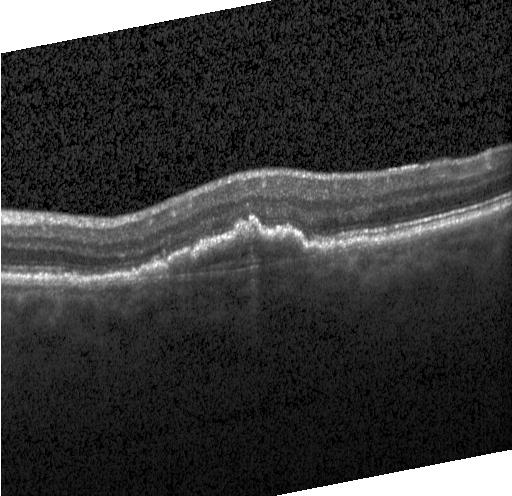 Retinal OCT cross-section.
Macular OCT: a choroidal neovascular membrane.